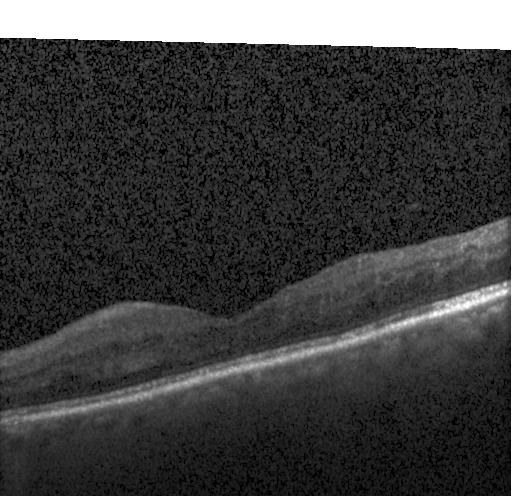 Finding: neither choroidal neovascularization, diabetic macular edema, nor drusen.